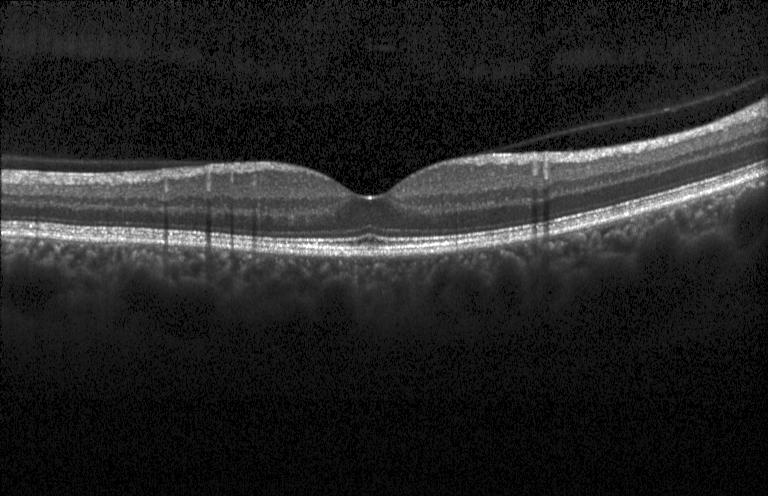 Retinal OCT B-scan. Centered on the fovea.
Diagnosis: no evidence of choroidal neovascularization, diabetic macular edema, or drusen.